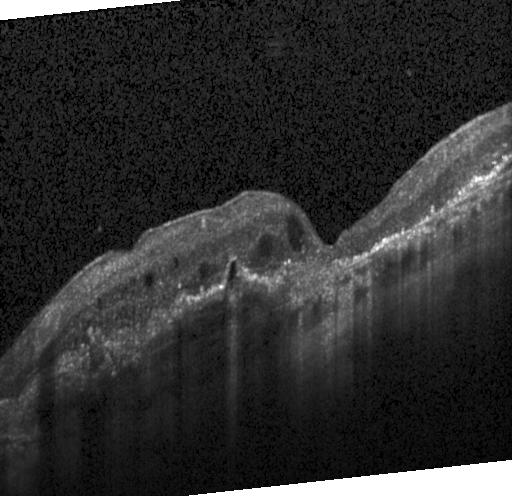 Retinal OCT B-scan, Heidelberg Spectralis, centered on the fovea.
OCT finding: choroidal neovascularization (CNV).